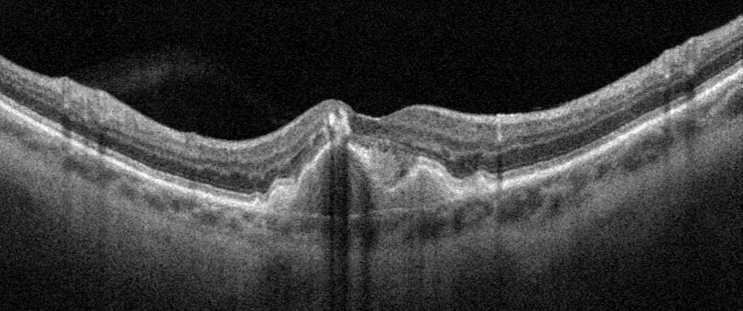
OCT B-scan showing AMD.